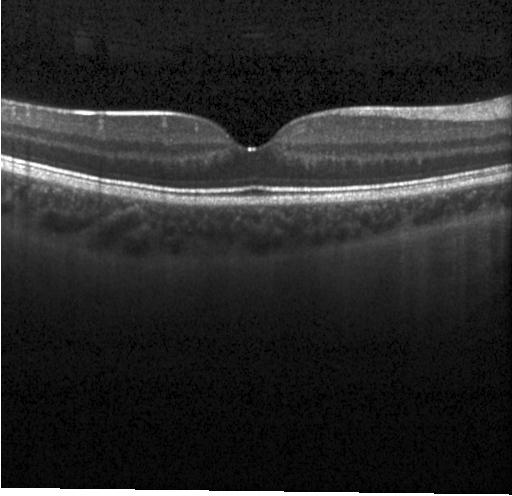 OCT B-scan · instrument: Heidelberg Spectralis · macular scan · SD-OCT.
Finding: no choroidal neovascularization, no diabetic macular edema, and no drusen.